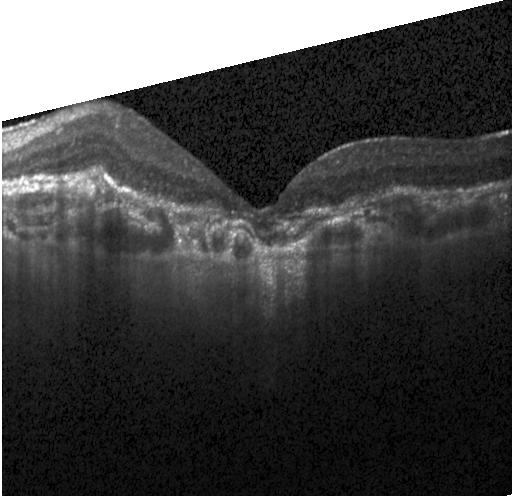
Heidelberg Spectralis OCT system. SD-OCT. Optical coherence tomography scan. Diagnosis: choroidal neovascularization.